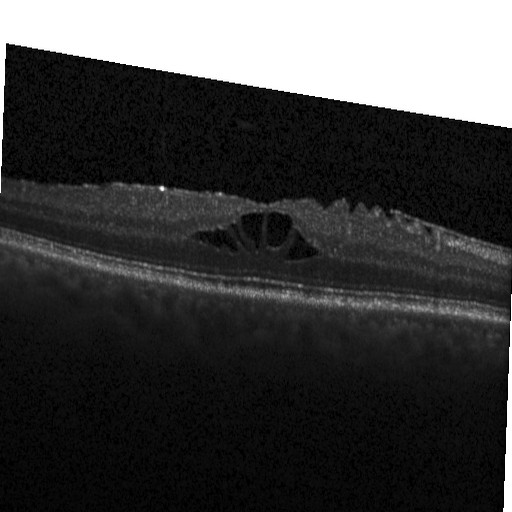
Macular scan. Optical coherence tomography B-scan. Spectral-domain optical coherence tomography. Heidelberg Spectralis.
Assessment: DME.